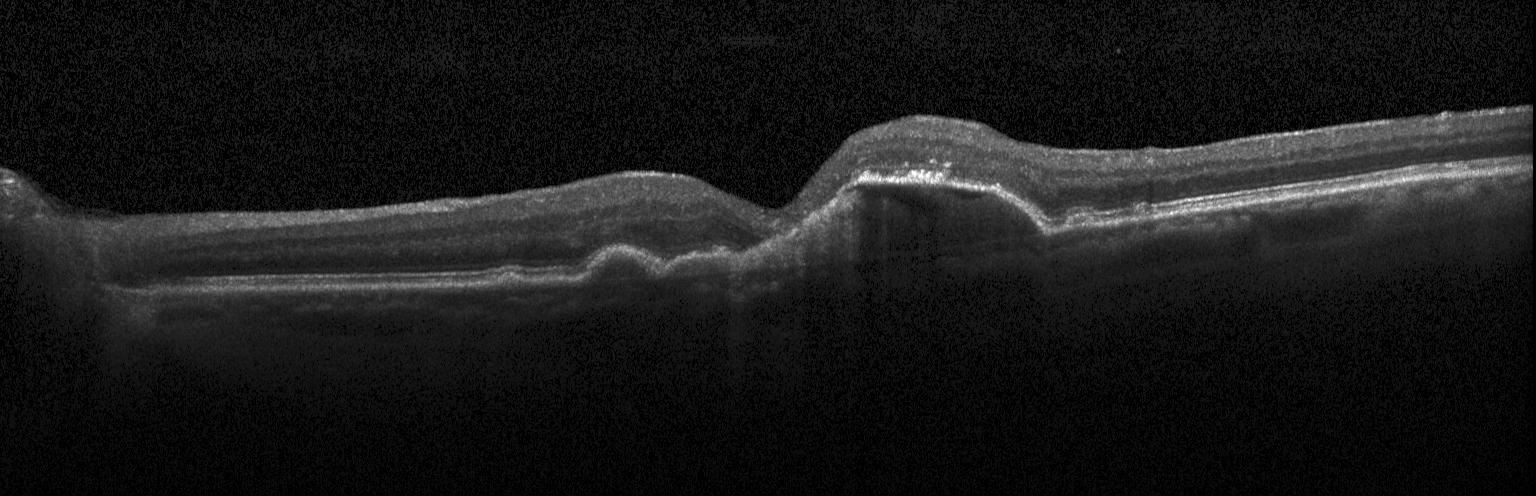

Heidelberg Spectralis, retinal OCT cross-section, macular scan — A choroidal neovascular membrane.